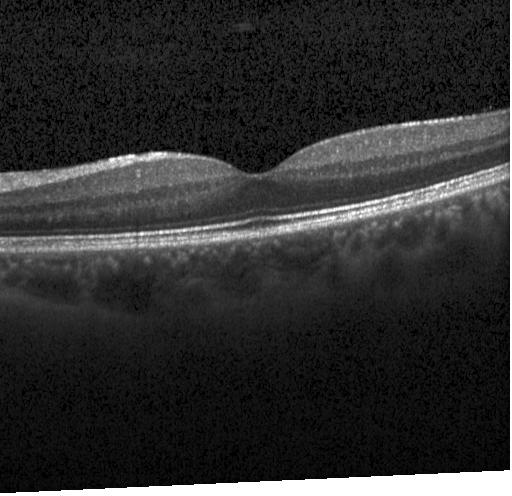
Retinal OCT cross-section. No choroidal neovascularization, diabetic macular edema, or drusen.